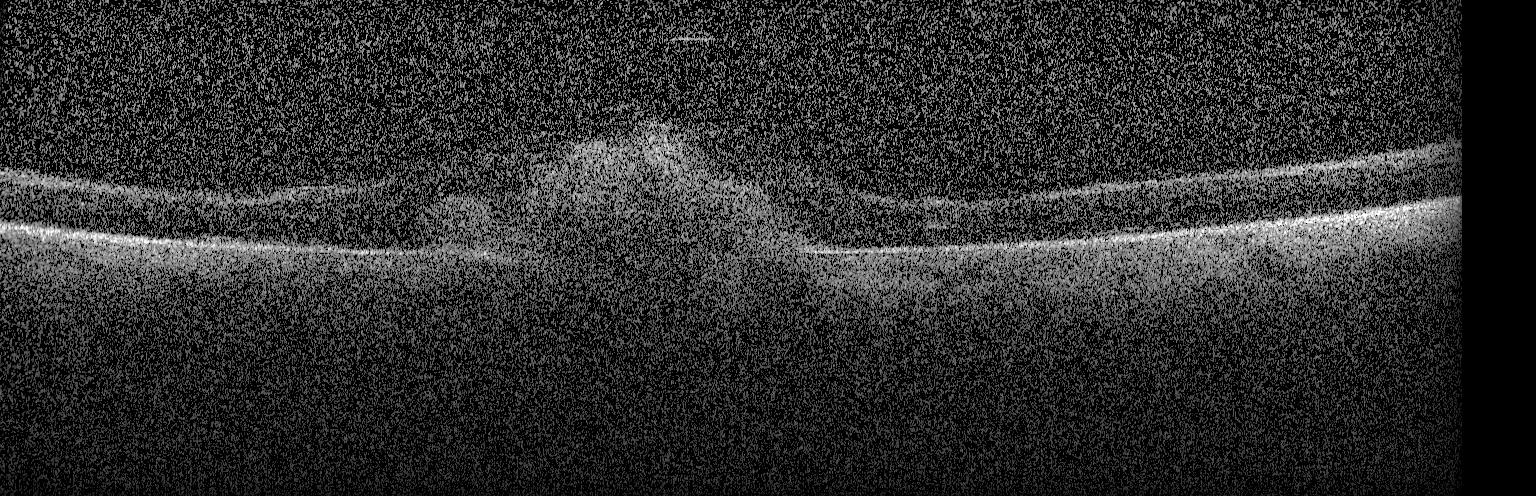
Impression: a choroidal neovascular membrane.